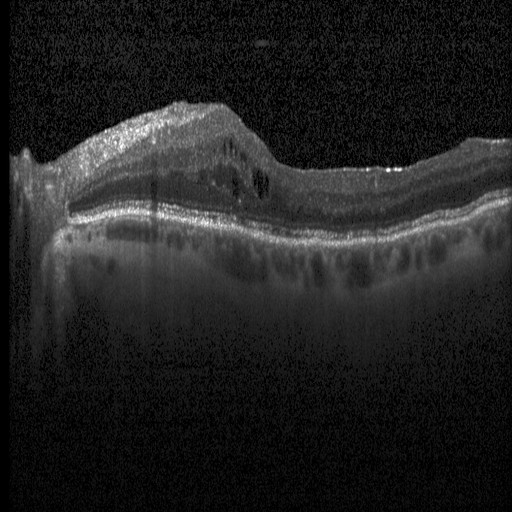

OCT line scan; spectral-domain OCT; acquired on a Heidelberg Spectralis; fovea-centered. Macular OCT: DME.